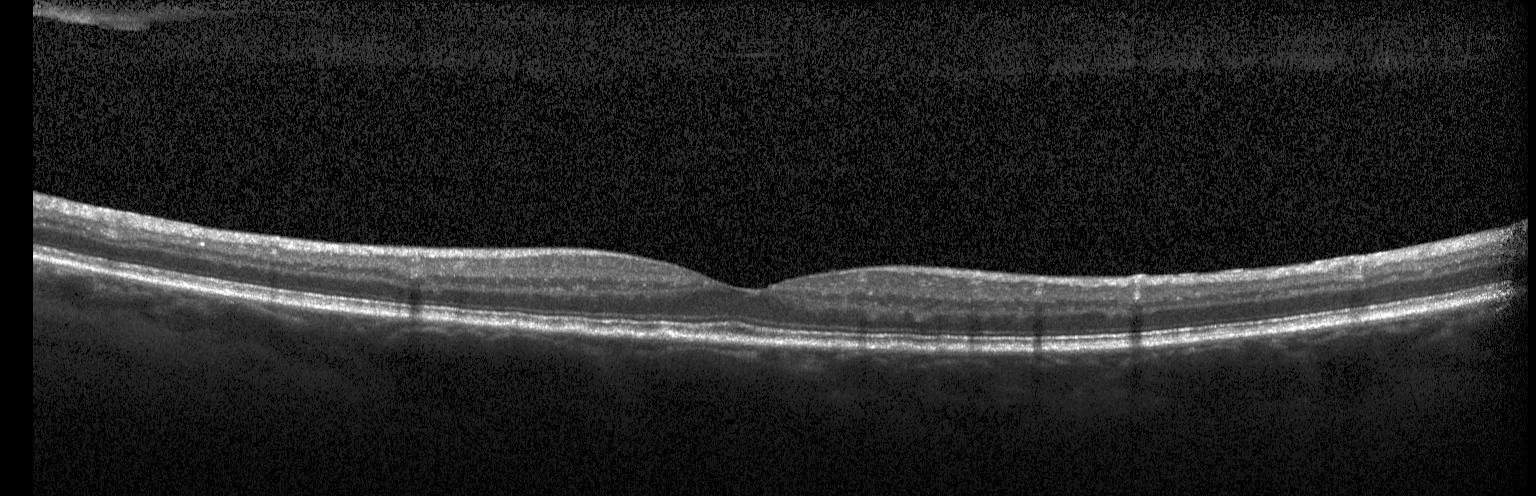

Optical coherence tomography B-scan. Heidelberg Spectralis OCT system
No choroidal neovascularization, no diabetic macular edema, and no drusen.